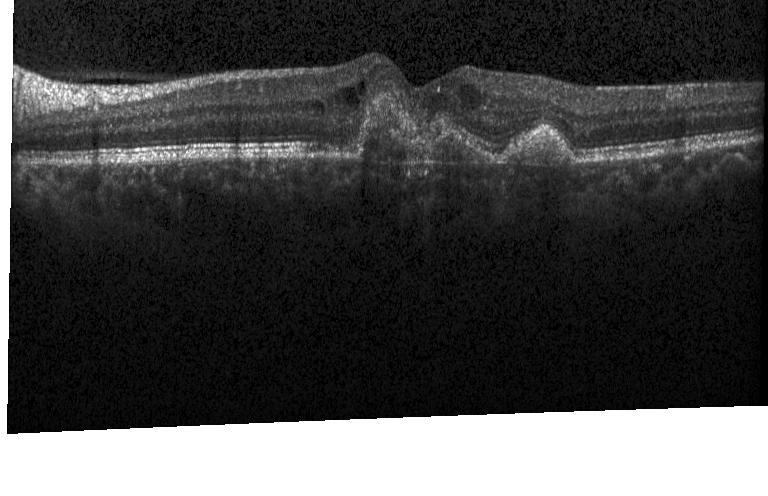
SD-OCT, retinal OCT cross-section, instrument: Heidelberg Spectralis
Assessment: a choroidal neovascular membrane.